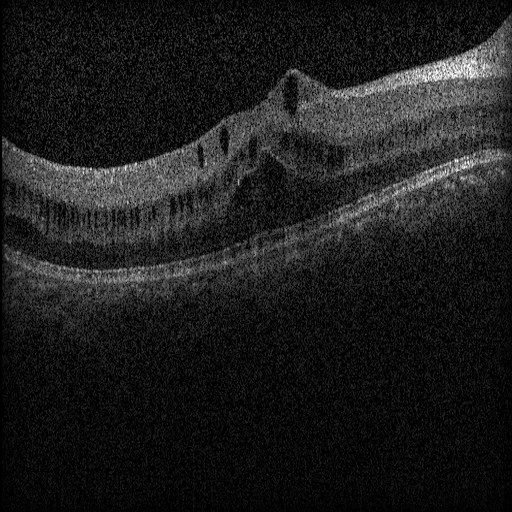
OCT B-scan showing DME.